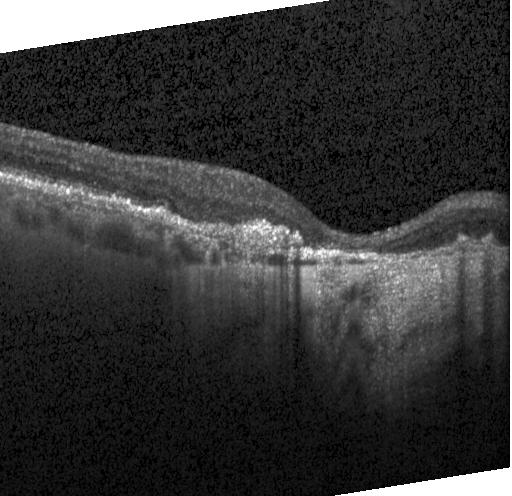
A choroidal neovascular membrane.